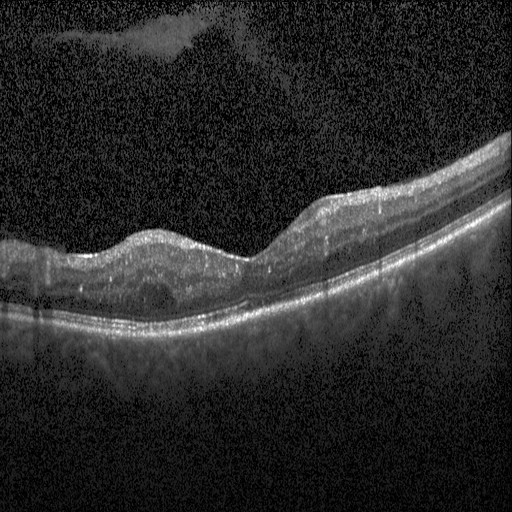 Diagnosis: DME.